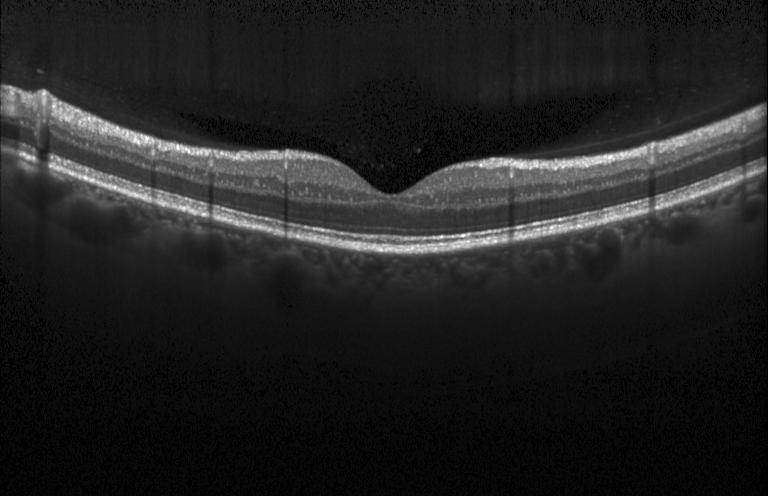
Through the macula. Heidelberg Spectralis. Retinal OCT B-scan — Neither choroidal neovascularization, diabetic macular edema, nor drusen.